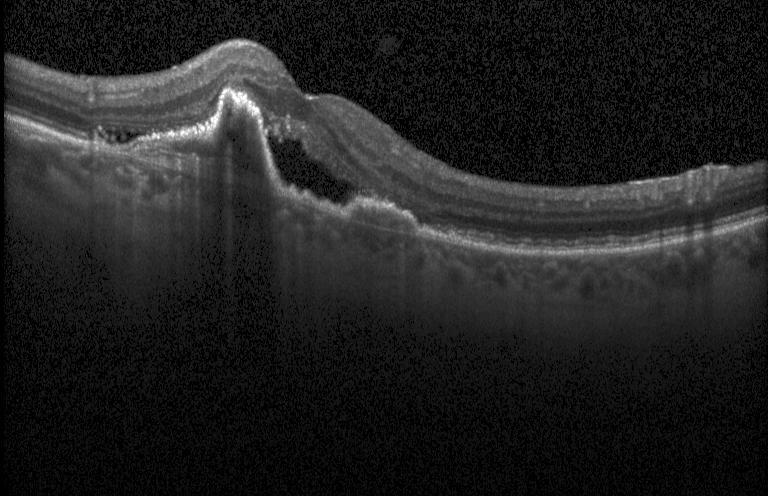

Retinal OCT B-scan
The scan shows choroidal neovascularization (CNV).